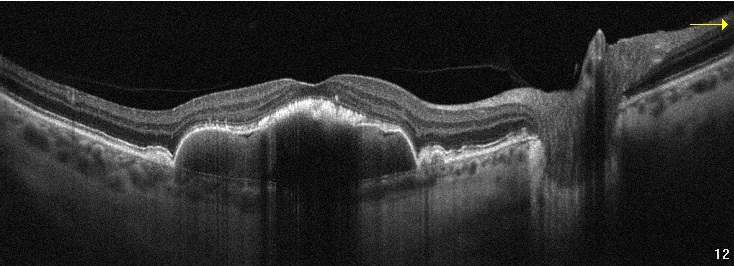 Optovue Avanti RTVue XR. OCT B-scan — OCT finding: AMD.